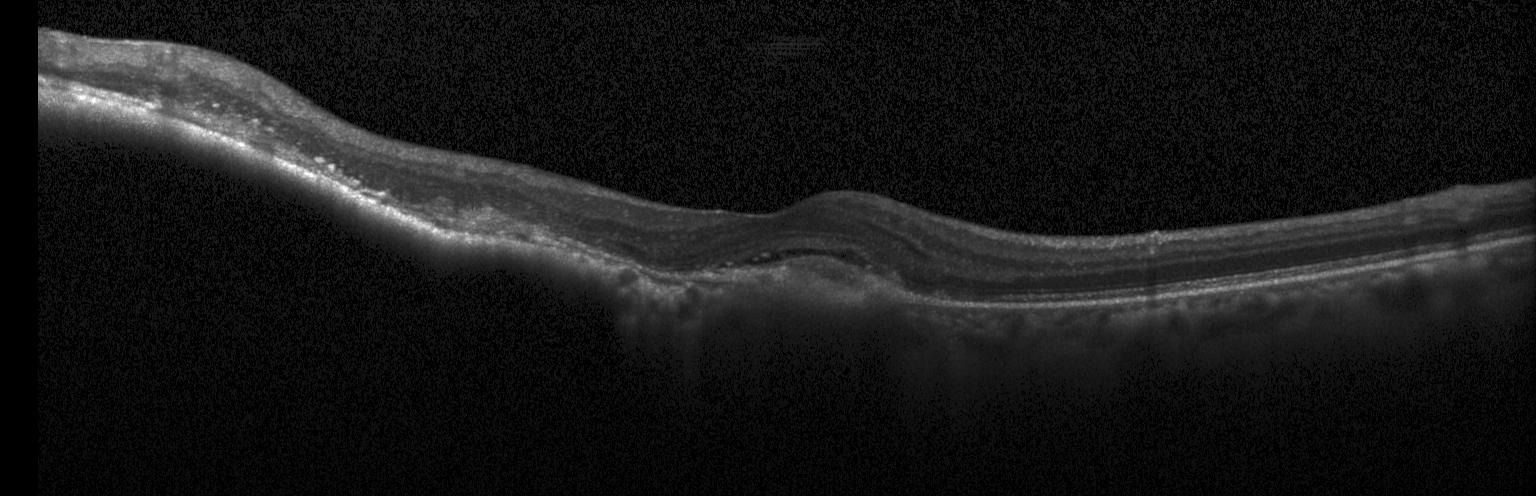
OCT line scan, centered on the fovea — Macular OCT: CNV.